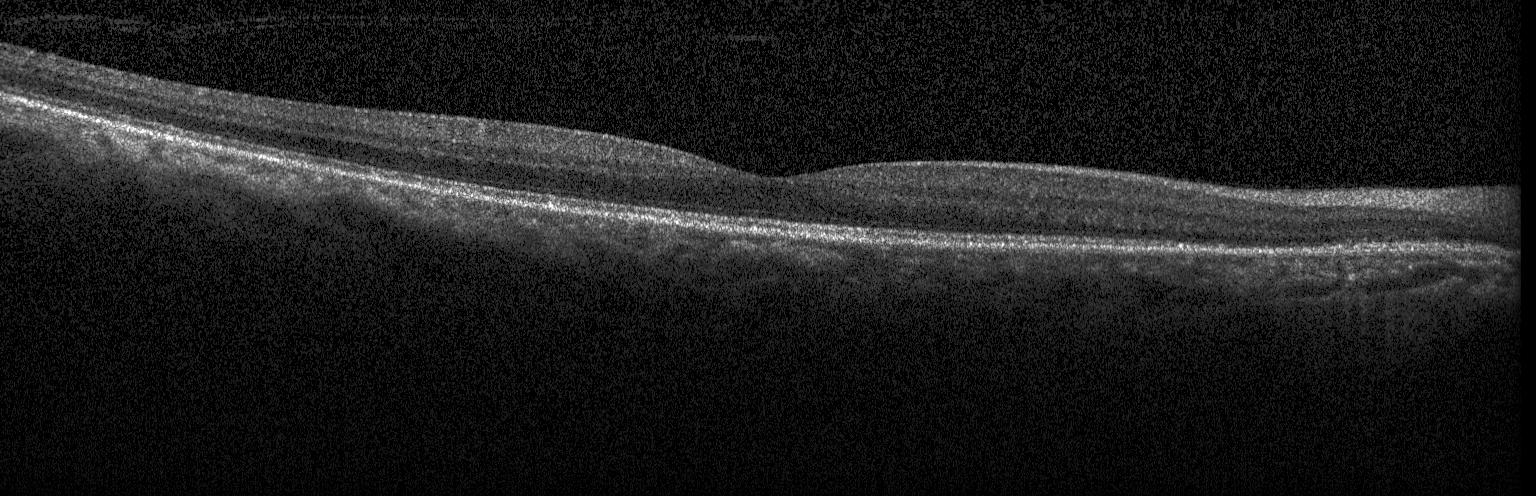 OCT line scan, spectral-domain optical coherence tomography, instrument: Heidelberg Spectralis
Diagnosis: no evidence of CNV, DME, or drusen.